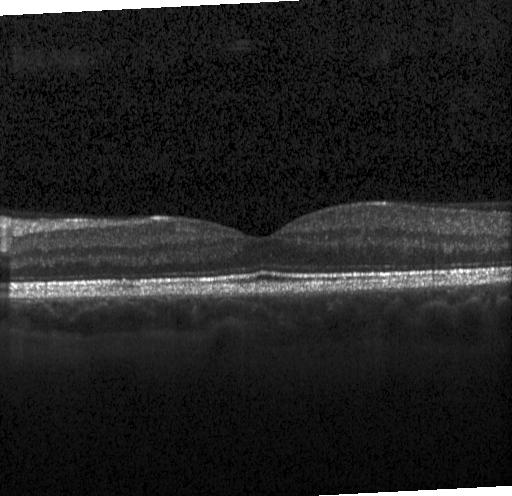
Optical coherence tomography B-scan — This B-scan demonstrates no choroidal neovascularization, no diabetic macular edema, and no drusen.